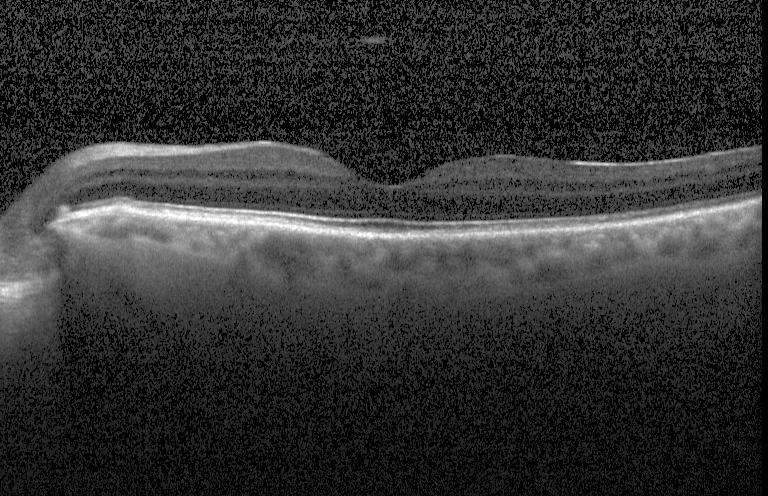
Optical coherence tomography scan, centered on the fovea, acquired on a Heidelberg Spectralis, SD-OCT.
Dx: no choroidal neovascularization, diabetic macular edema, or drusen.